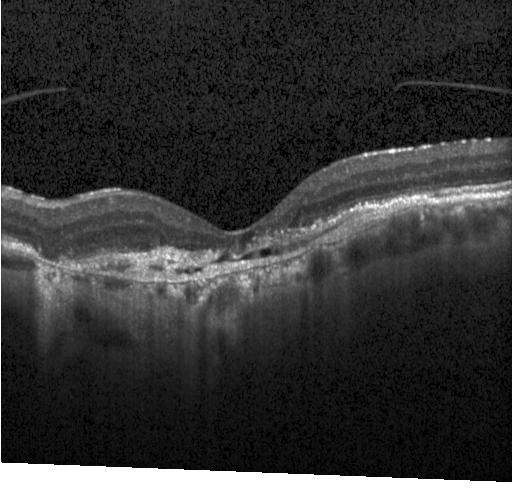

Dx: a choroidal neovascular membrane.